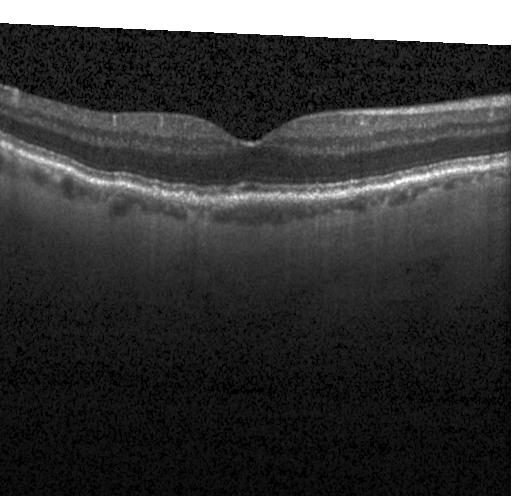

Diagnosis: drusen.